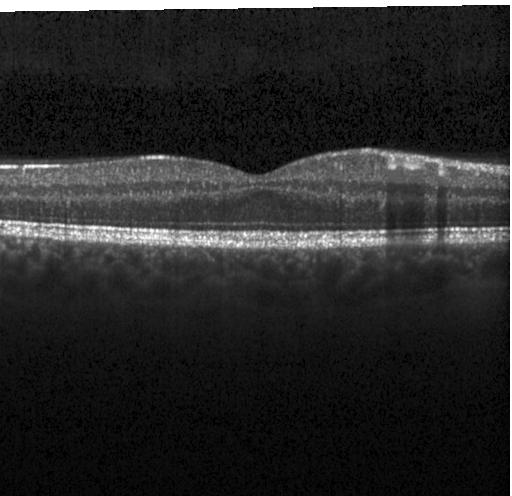

Spectral-domain optical coherence tomography; macular scan; acquired on a Heidelberg Spectralis; OCT B-scan
Impression: no CNV, no DME, and no drusen.